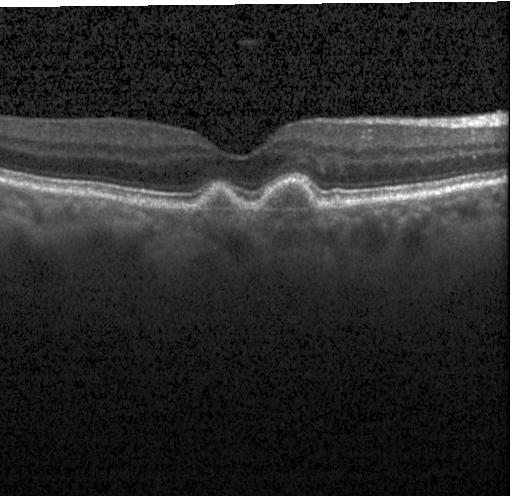

Optical coherence tomography B-scan; acquired on a Heidelberg Spectralis
OCT finding: drusen.